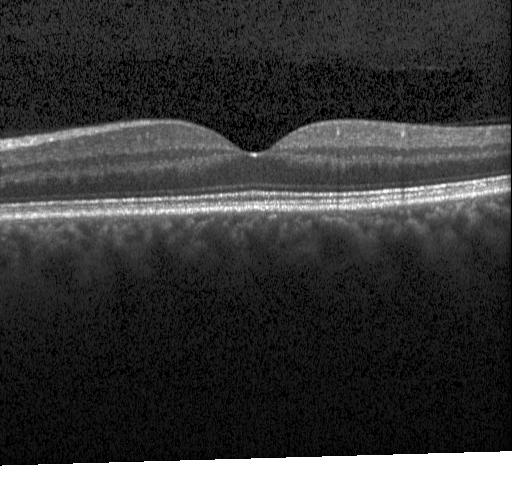
Optical coherence tomography B-scan. Through the macula
Diagnosis: no choroidal neovascularization, diabetic macular edema, or drusen.